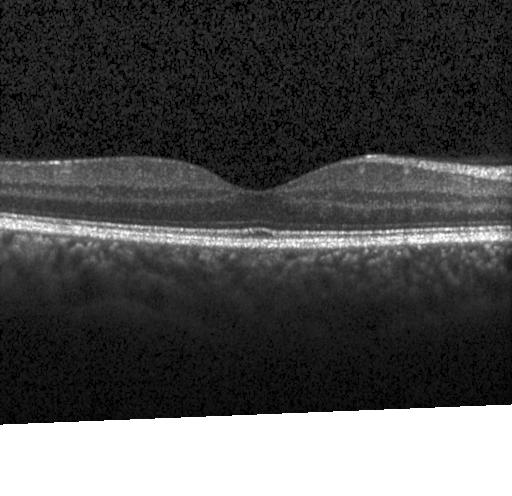
Dx: no choroidal neovascularization, no diabetic macular edema, and no drusen.